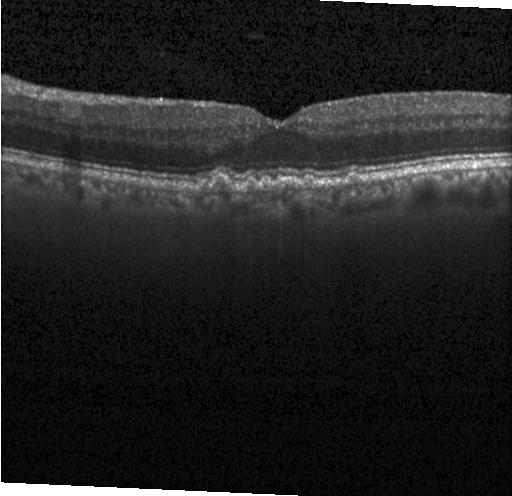

OCT line scan
Macular OCT: multiple drusen.